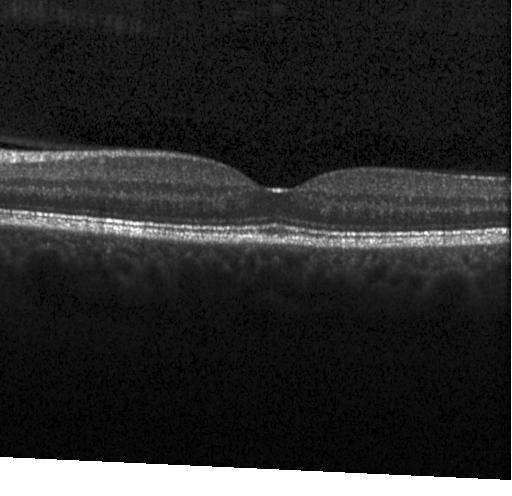
Impression: no CNV, DME, or drusen.